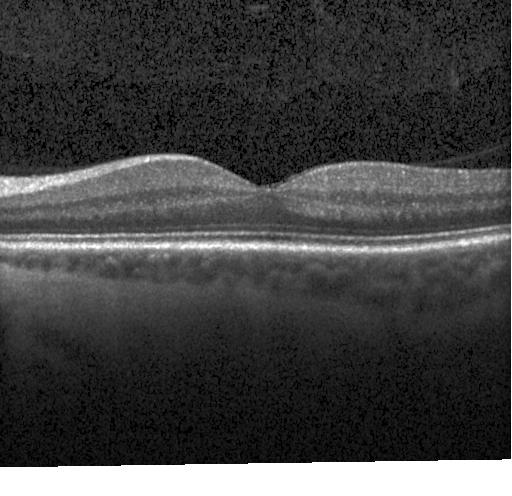

The scan shows no choroidal neovascularization, diabetic macular edema, or drusen.